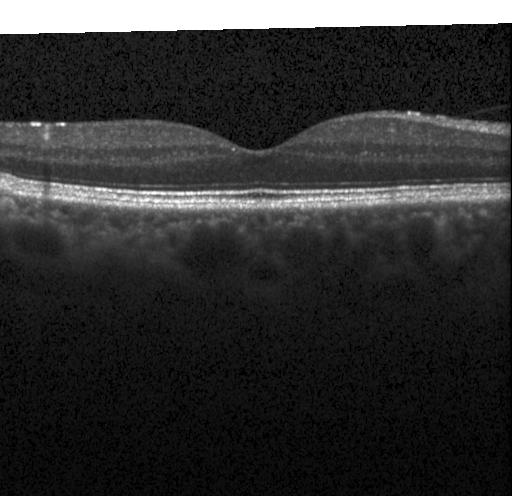
OCT B-scan
Dx: no evidence of choroidal neovascularization, diabetic macular edema, or drusen.